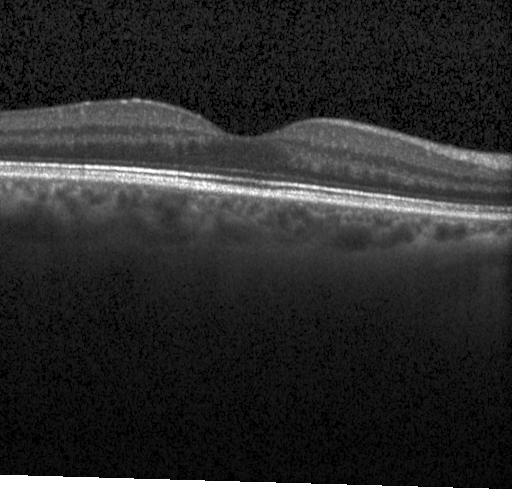
Horizontal scan through the fovea · instrument: Heidelberg Spectralis · OCT line scan. Impression: neither CNV, DME, nor drusen.